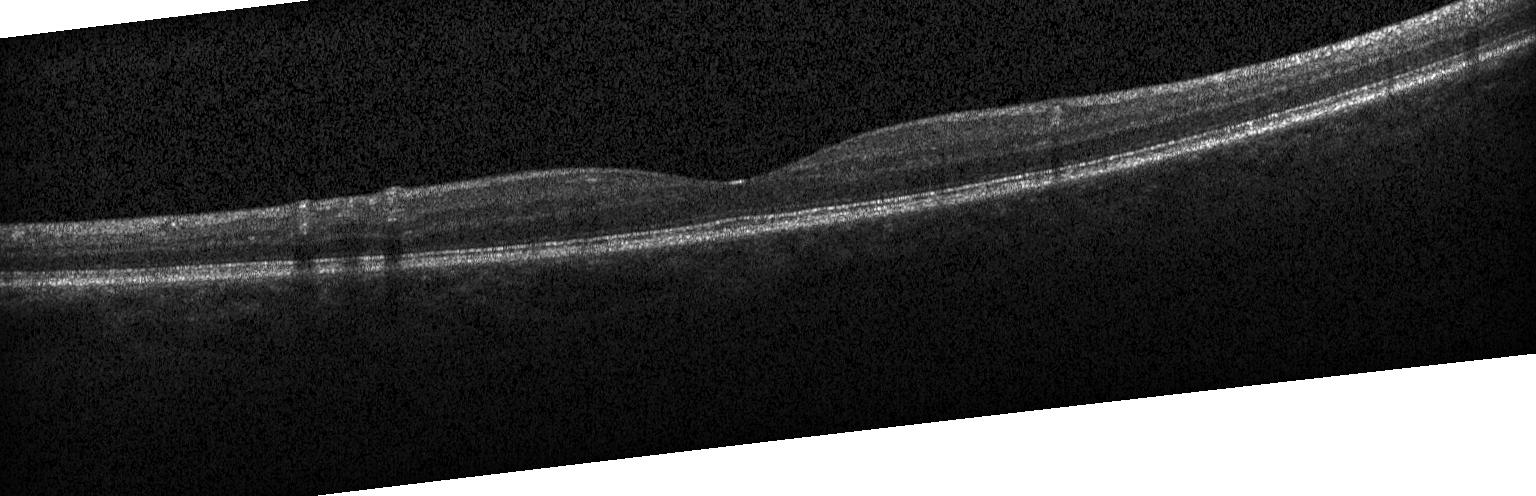 OCT scan showing no choroidal neovascularization, no diabetic macular edema, and no drusen.